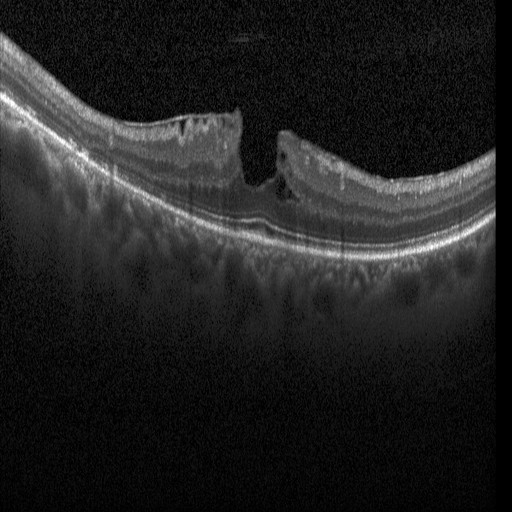 Retinal OCT B-scan
This B-scan demonstrates diabetic macular edema.